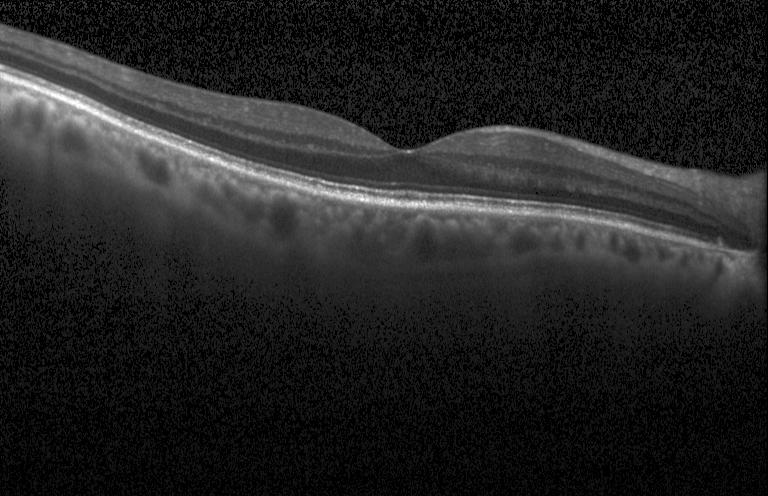

Centered on the fovea. Instrument: Heidelberg Spectralis. Optical coherence tomography scan. The scan shows no CNV, DME, or drusen.